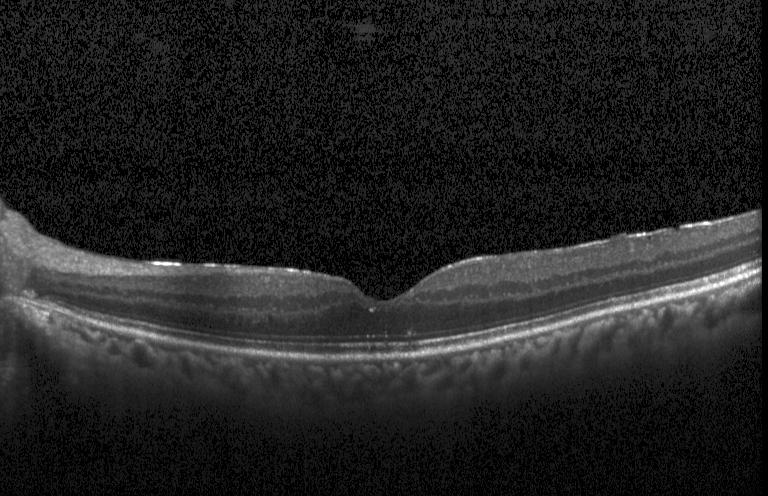
Centered on the fovea, SD-OCT, OCT B-scan — Impression: no evidence of CNV, DME, or drusen.